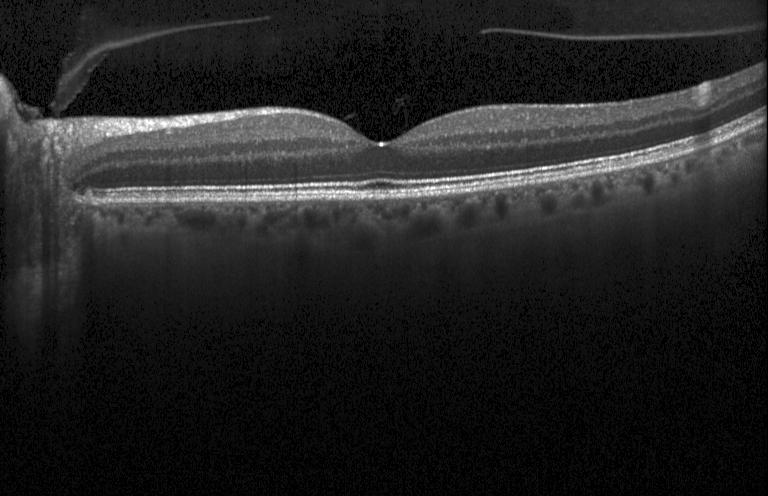
Diagnosis: neither choroidal neovascularization, diabetic macular edema, nor drusen.